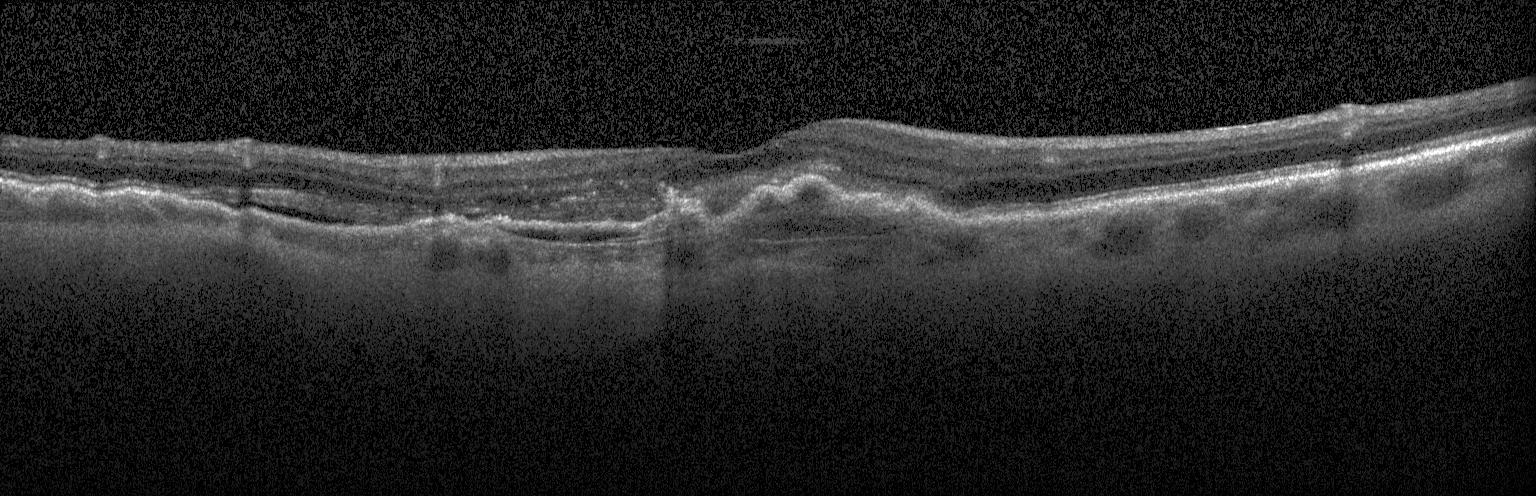
Retinal OCT B-scan; Heidelberg Spectralis; through the macula — Assessment: a choroidal neovascular membrane.